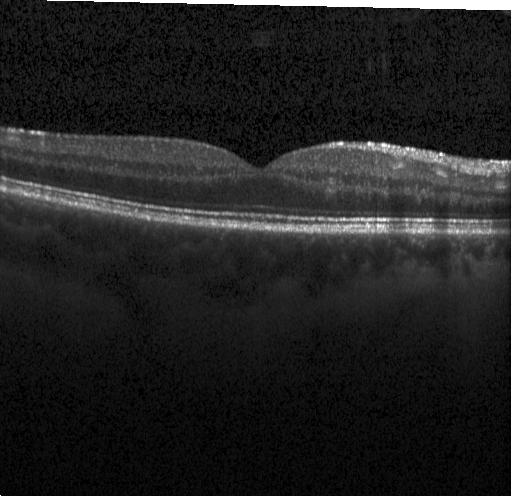

Macular OCT demonstrating no choroidal neovascularization, diabetic macular edema, or drusen.